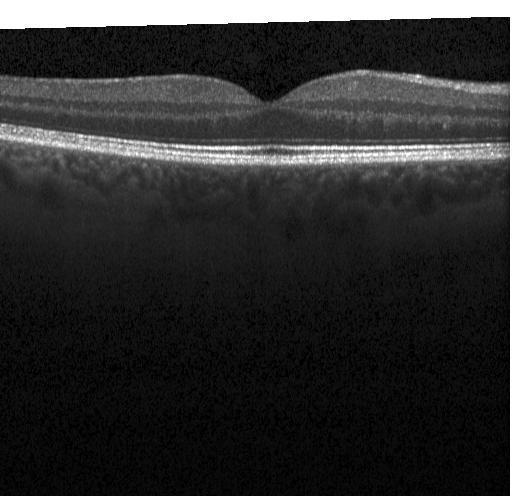
Heidelberg Spectralis. Retinal OCT cross-section.
Impression: no evidence of CNV, DME, or drusen.